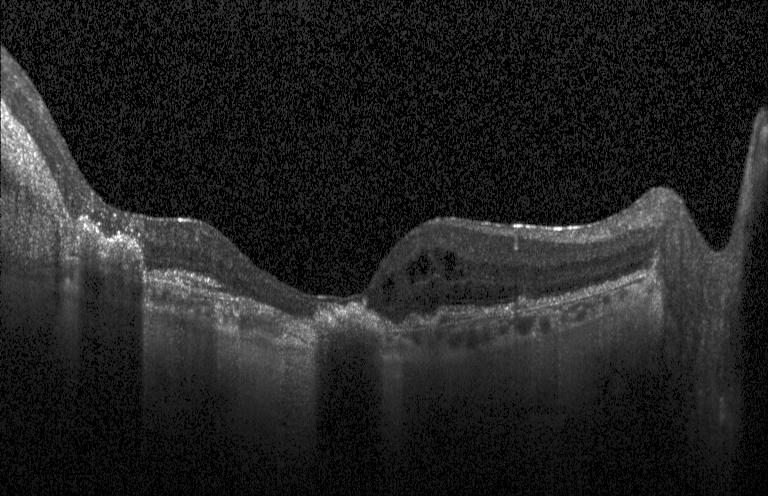

OCT scan showing choroidal neovascularization.